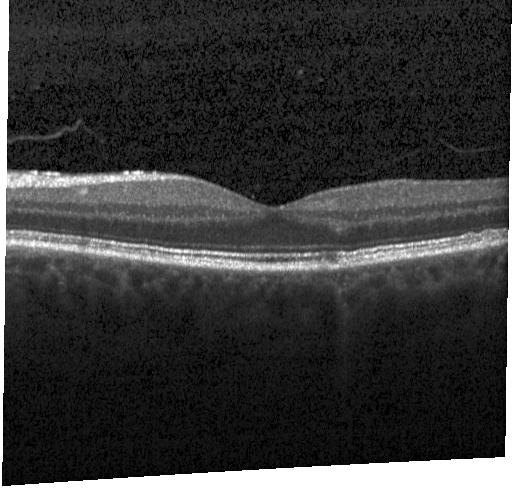 Macular OCT: no choroidal neovascularization, no diabetic macular edema, and no drusen.